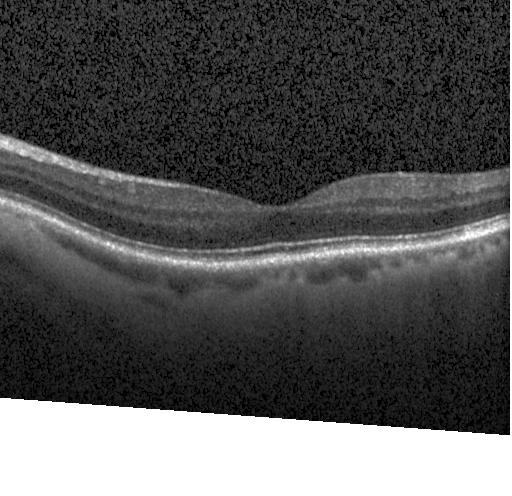
OCT B-scan; acquired on a Heidelberg Spectralis. No choroidal neovascularization, diabetic macular edema, or drusen.